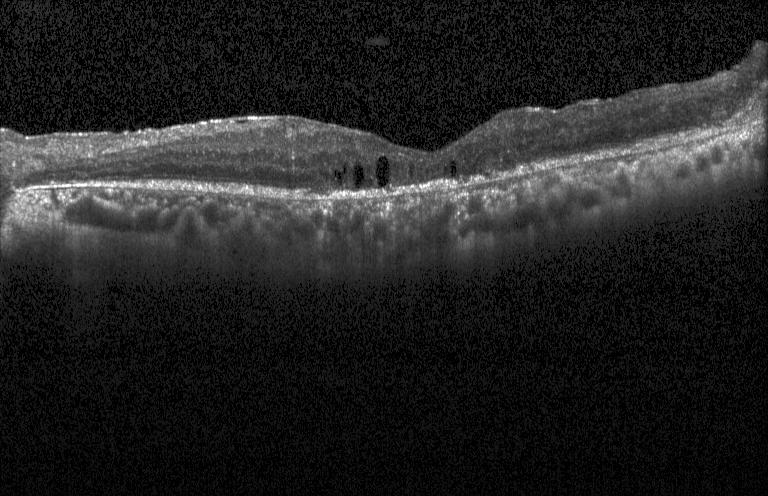 OCT line scan; SD-OCT; fovea-centered; acquired on a Heidelberg Spectralis
Assessment: choroidal neovascularization (CNV).